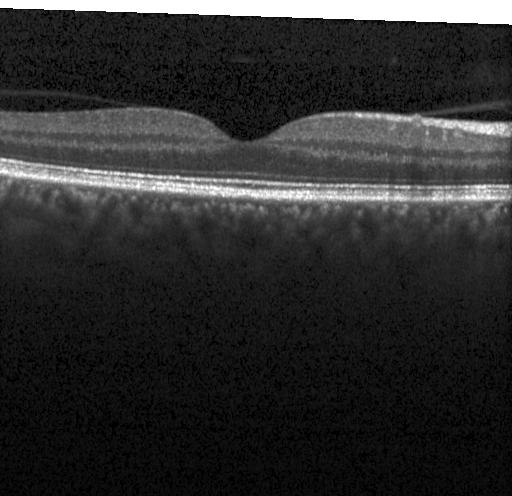

Fovea-centered; instrument: Heidelberg Spectralis; SD-OCT; OCT B-scan — Dx: no choroidal neovascularization, no diabetic macular edema, and no drusen.